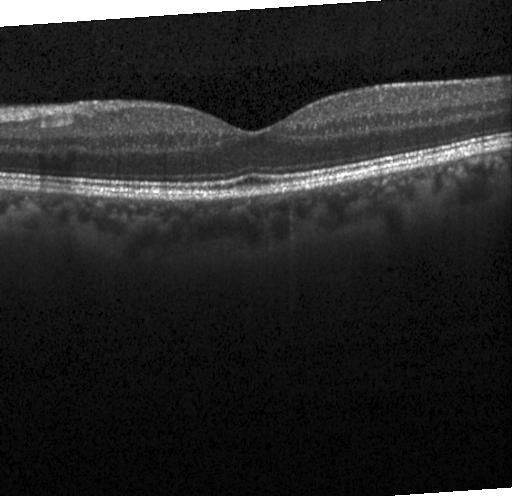
Heidelberg Spectralis OCT system; optical coherence tomography scan; spectral-domain OCT; macular scan
OCT finding: no choroidal neovascularization, no diabetic macular edema, and no drusen.